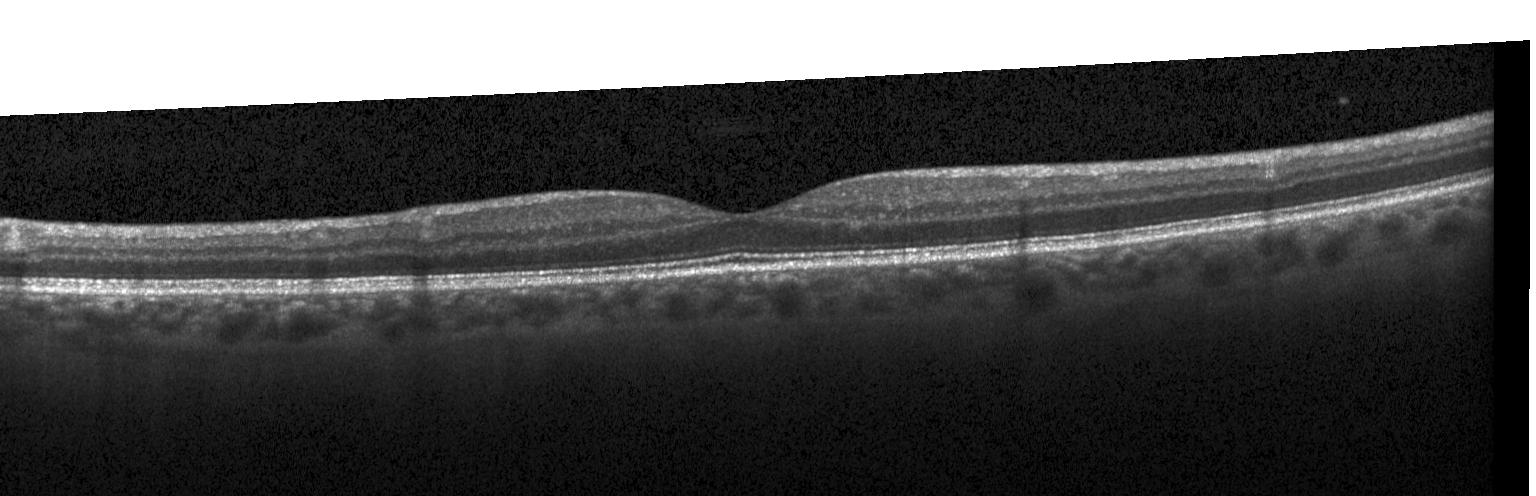

Retinal OCT cross-section showing no evidence of choroidal neovascularization, diabetic macular edema, or drusen.